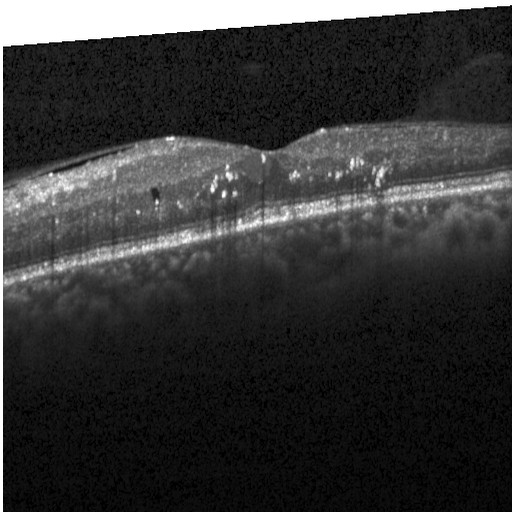

Optical coherence tomography B-scan; spectral-domain OCT; through the macula; Heidelberg Spectralis.
The scan shows diabetic macular edema.